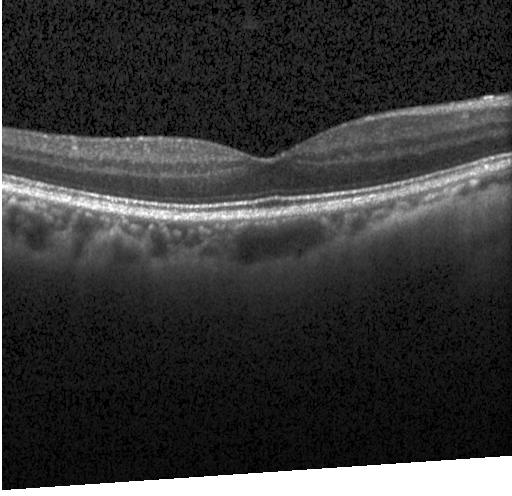
Retinal OCT cross-section.
Dx: no choroidal neovascularization, no diabetic macular edema, and no drusen.